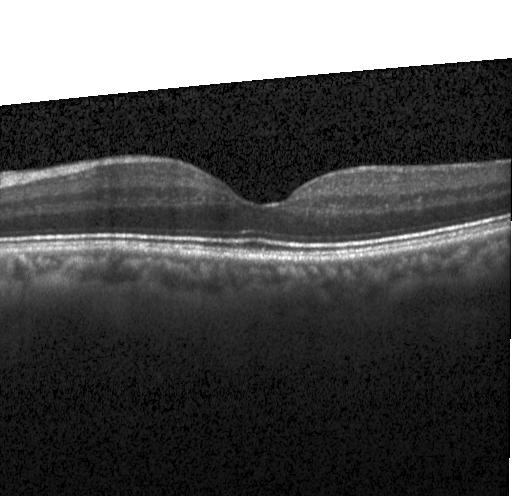 Optical coherence tomography B-scan, spectral-domain optical coherence tomography — Diagnosis: no choroidal neovascularization, diabetic macular edema, or drusen.